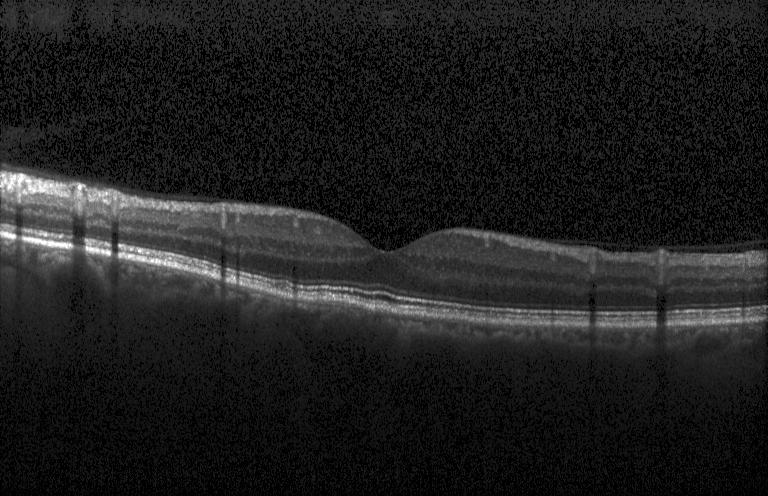
This B-scan demonstrates no evidence of CNV, DME, or drusen.